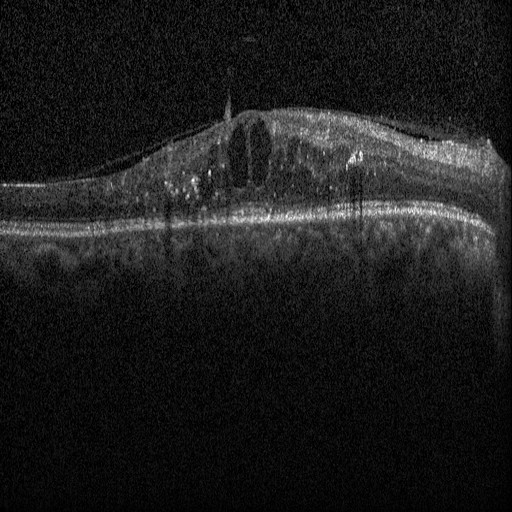
Retinal OCT cross-section. Finding: DME.